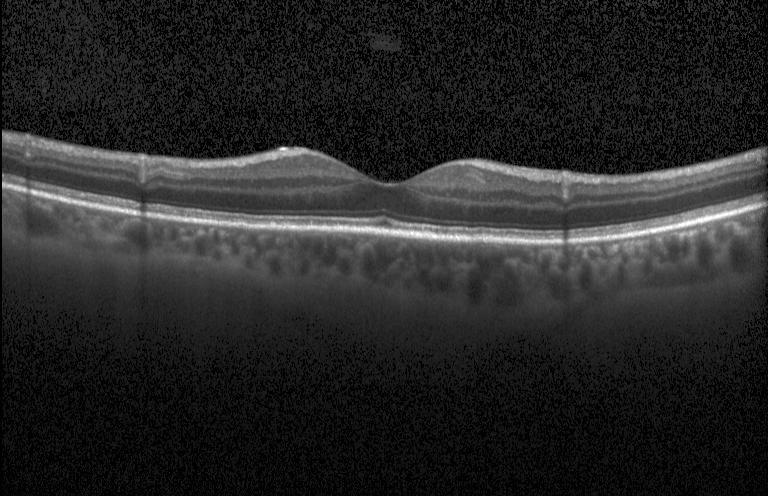 OCT B-scan, acquired on a Heidelberg Spectralis, macular scan. This B-scan demonstrates no choroidal neovascularization, no diabetic macular edema, and no drusen.